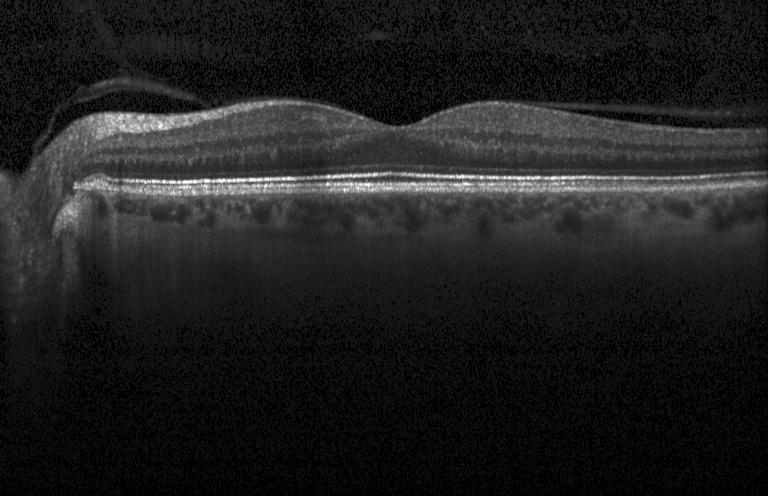

Heidelberg Spectralis, SD-OCT, optical coherence tomography B-scan, centered on the fovea. Finding: neither CNV, DME, nor drusen.